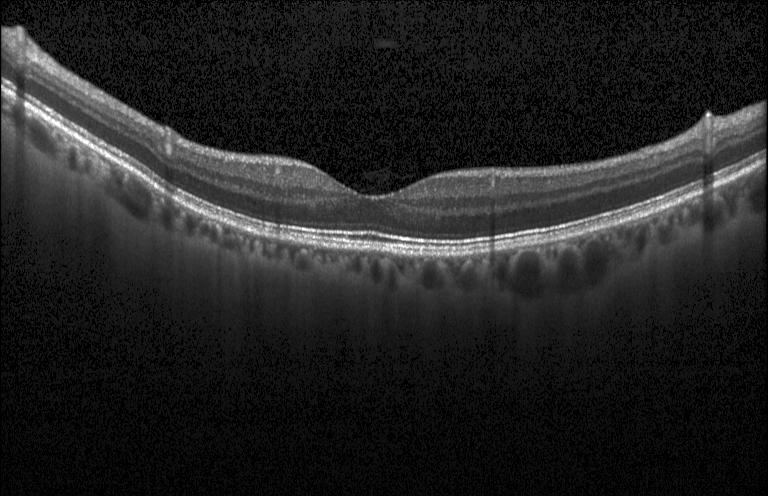
Retinal OCT cross-section — This B-scan demonstrates no choroidal neovascularization, diabetic macular edema, or drusen.